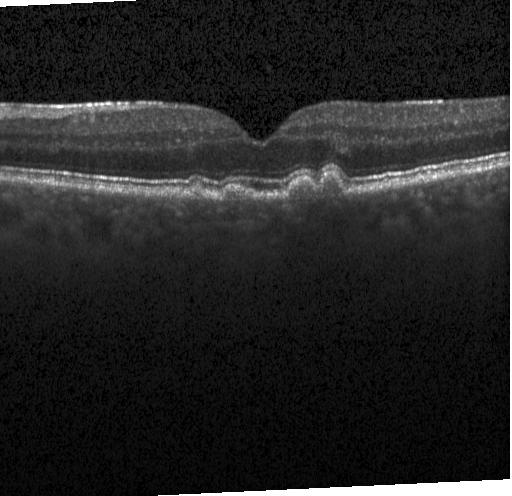

Optical coherence tomography scan — The scan shows sub-RPE drusenoid deposits.